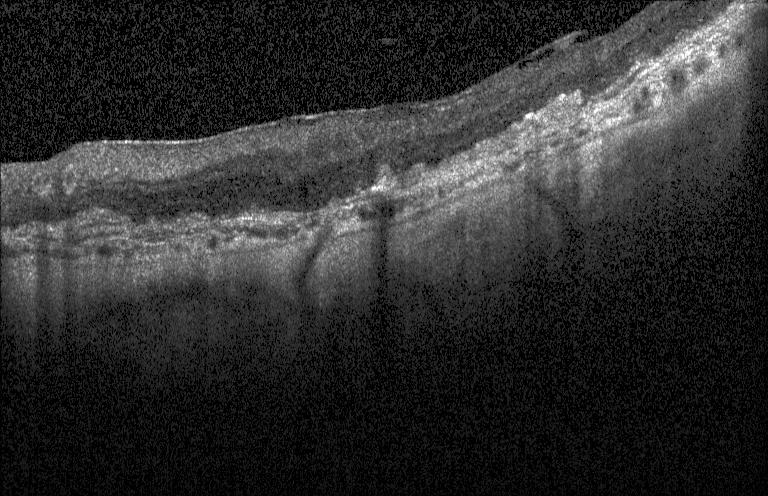
Optical coherence tomography scan. Diagnosis: a choroidal neovascular membrane.